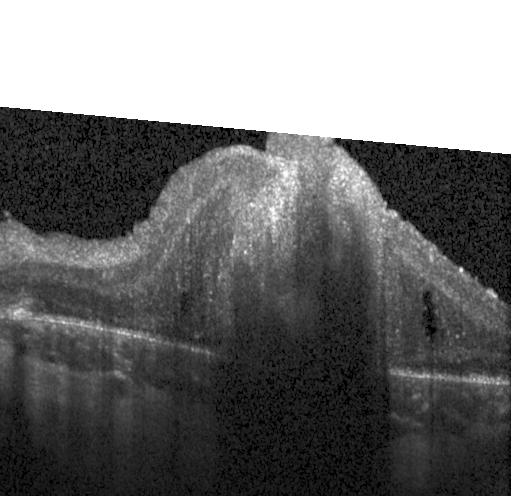
Macular OCT: choroidal neovascularization (CNV).